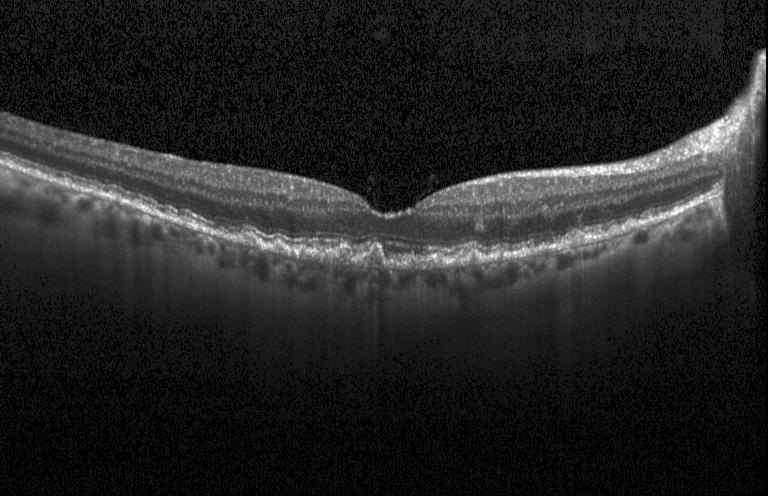

Horizontal scan through the fovea, retinal OCT B-scan.
Finding: sub-RPE drusenoid deposits.